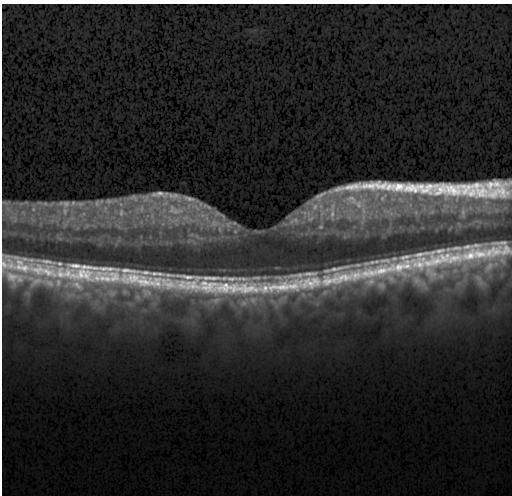 Acquired on a Heidelberg Spectralis, retinal OCT B-scan
Diagnosis: no choroidal neovascularization, diabetic macular edema, or drusen.